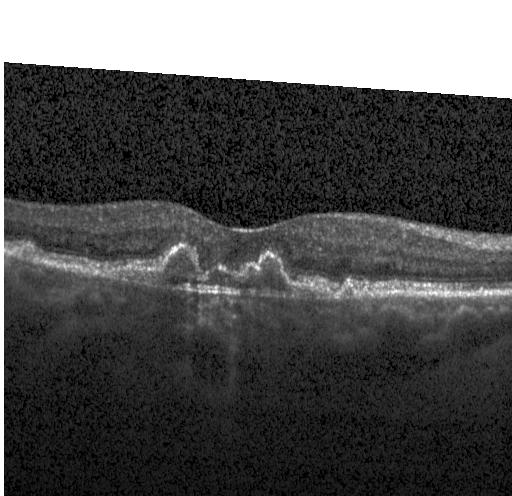 OCT B-scan — Diagnosis: a choroidal neovascular membrane.